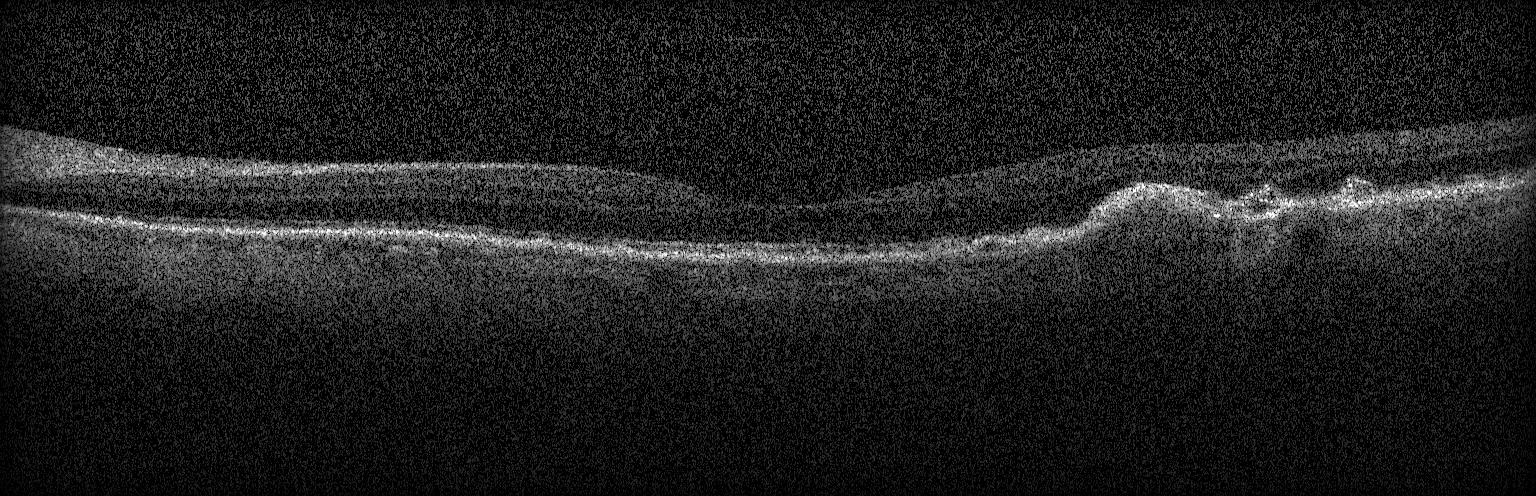 Dx: a choroidal neovascular membrane.